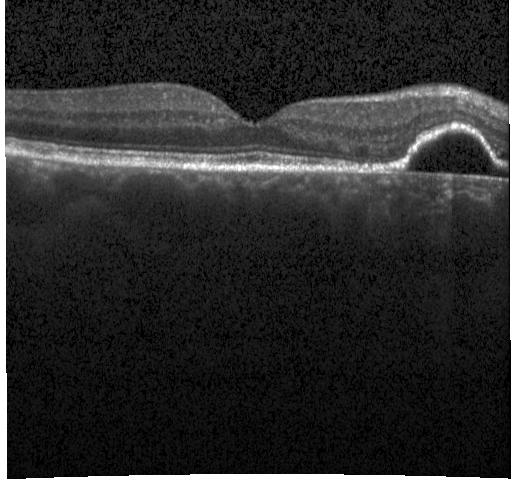

Spectral-domain OCT B-scan: choroidal neovascularization.